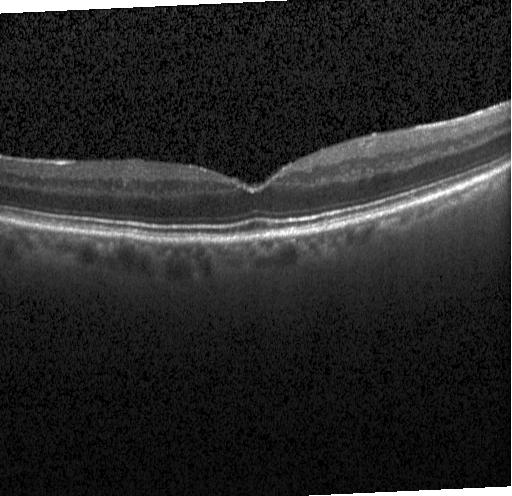 The scan shows no choroidal neovascularization, no diabetic macular edema, and no drusen.